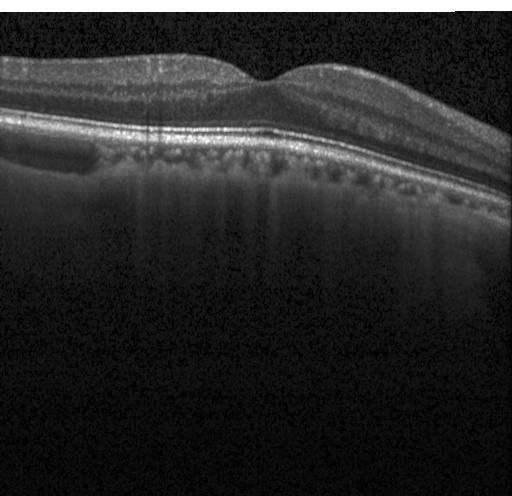
Impression: neither choroidal neovascularization, diabetic macular edema, nor drusen.